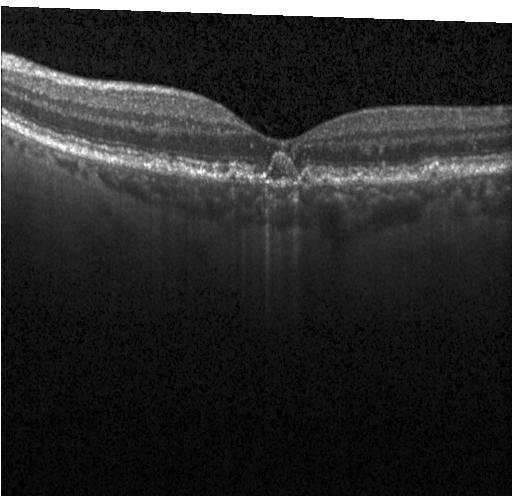
OCT finding: choroidal neovascularization (CNV).